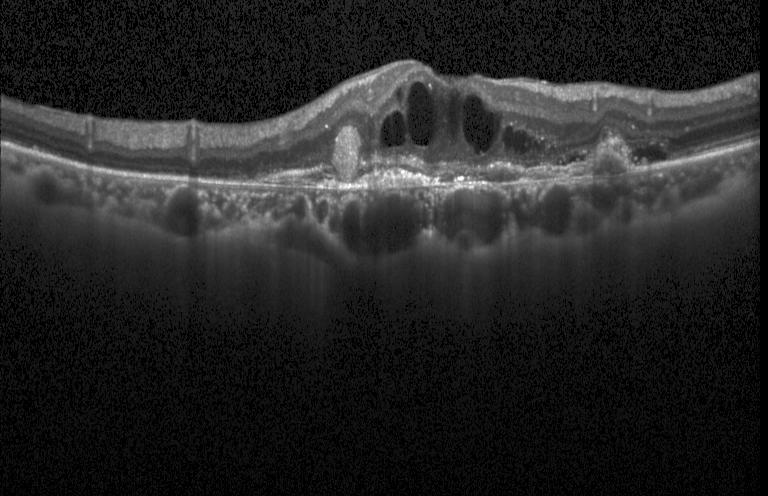 OCT line scan · fovea-centered · Heidelberg Spectralis OCT system.
Macular OCT: a choroidal neovascular membrane.